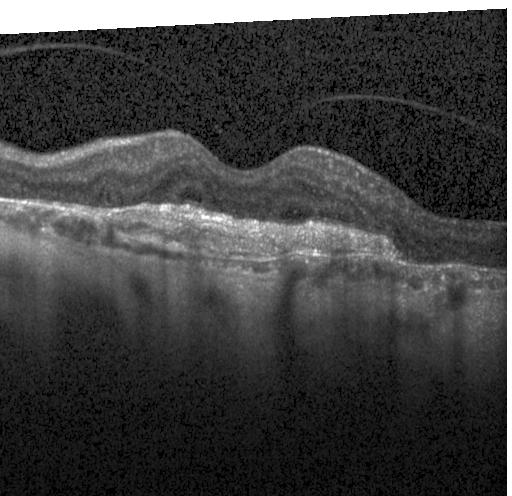
Heidelberg Spectralis. Spectral-domain OCT. OCT B-scan. Horizontal scan through the fovea — Finding: choroidal neovascularization (CNV).